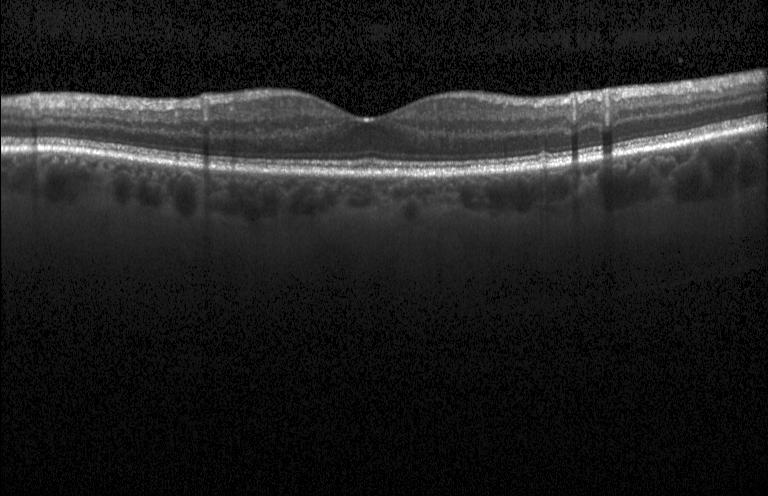
Macular OCT demonstrating neither choroidal neovascularization, diabetic macular edema, nor drusen.